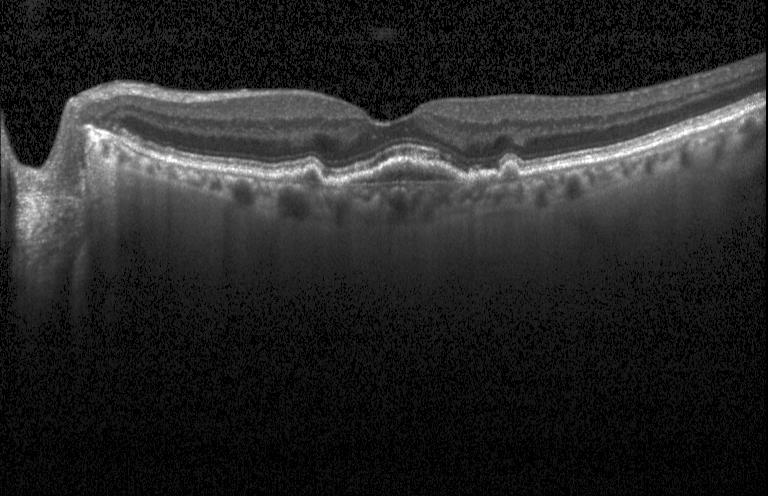

Retinal OCT cross-section — Diagnosis: a choroidal neovascular membrane.